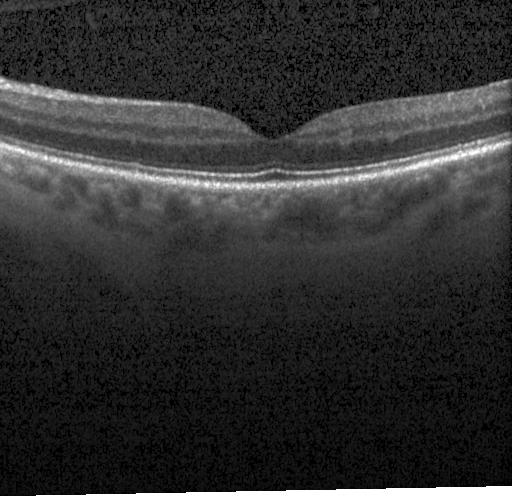
Retinal OCT cross-section; macular scan — Finding: no choroidal neovascularization, no diabetic macular edema, and no drusen.